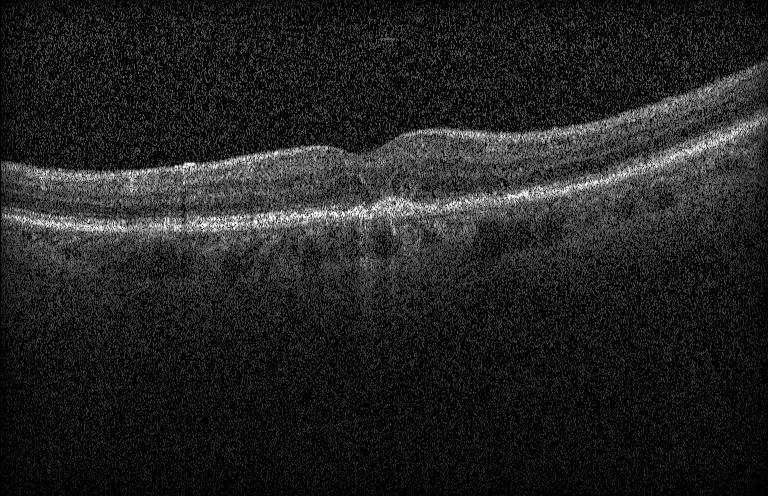
Diagnosis: a choroidal neovascular membrane.